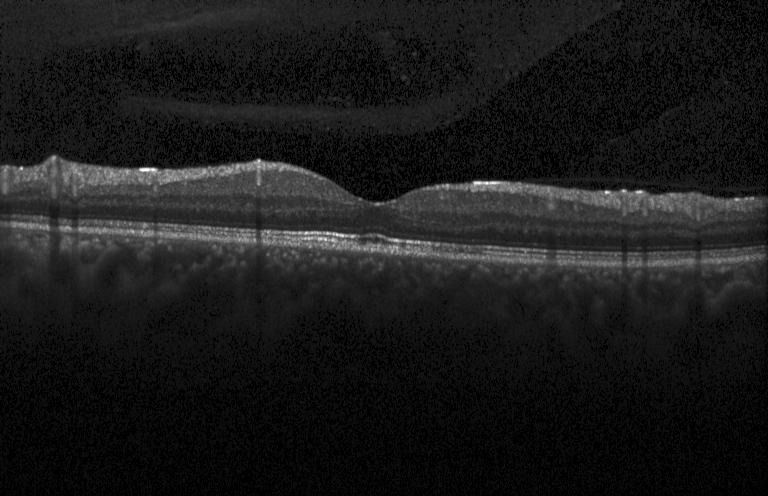
Macular OCT: neither choroidal neovascularization, diabetic macular edema, nor drusen.